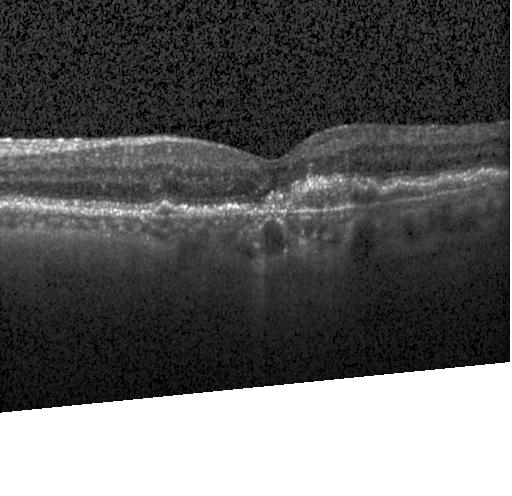

OCT line scan, macular scan, Heidelberg Spectralis OCT system, SD-OCT — Finding: choroidal neovascularization (CNV).